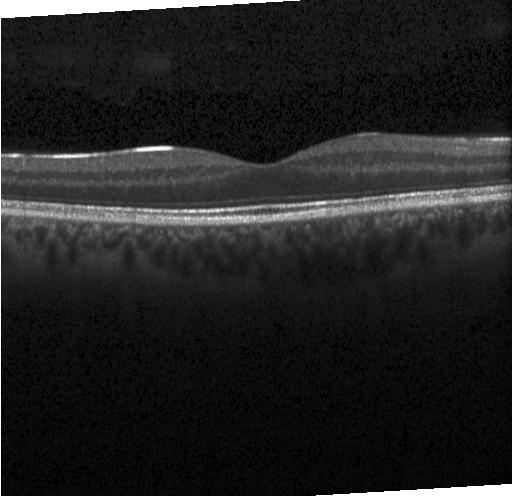

OCT line scan
Finding: neither choroidal neovascularization, diabetic macular edema, nor drusen.